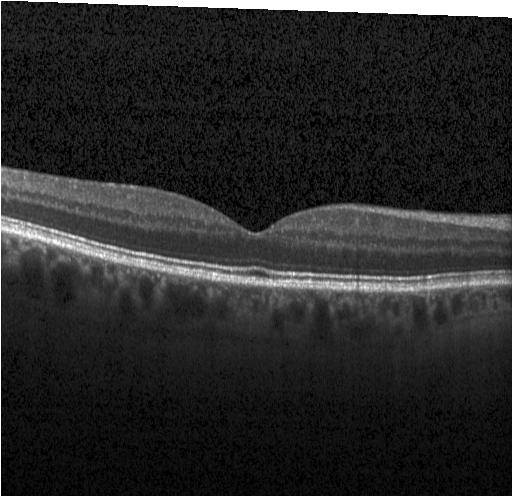
Spectral-domain optical coherence tomography · optical coherence tomography scan · instrument: Heidelberg Spectralis · horizontal scan through the fovea.
No evidence of choroidal neovascularization, diabetic macular edema, or drusen.